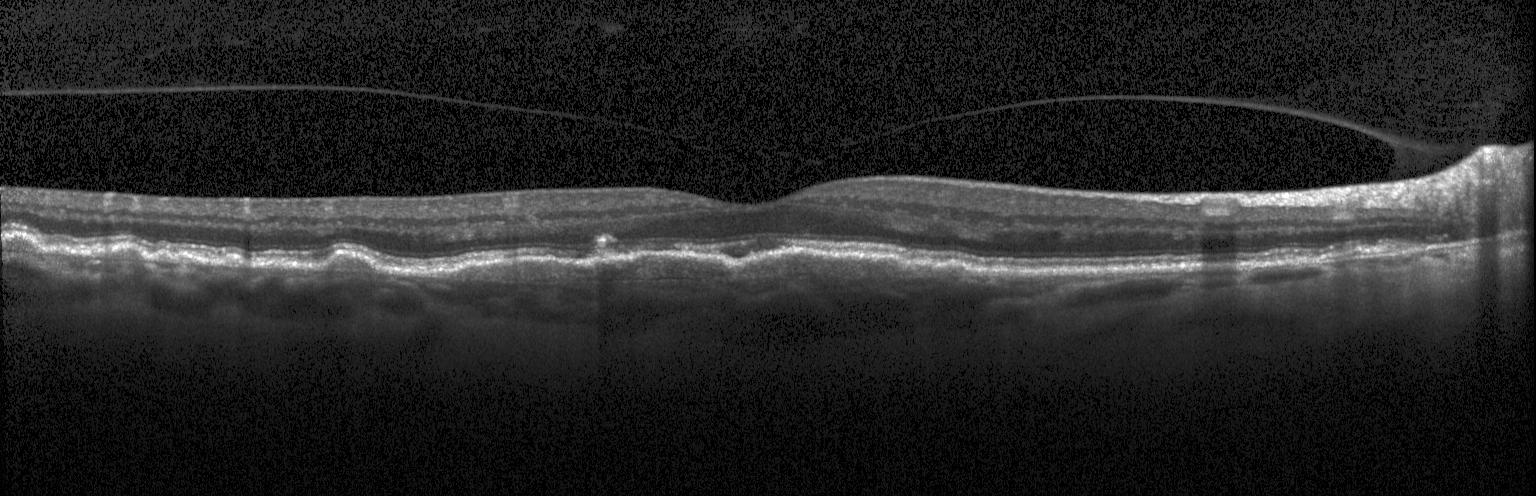
This B-scan demonstrates choroidal neovascularization.